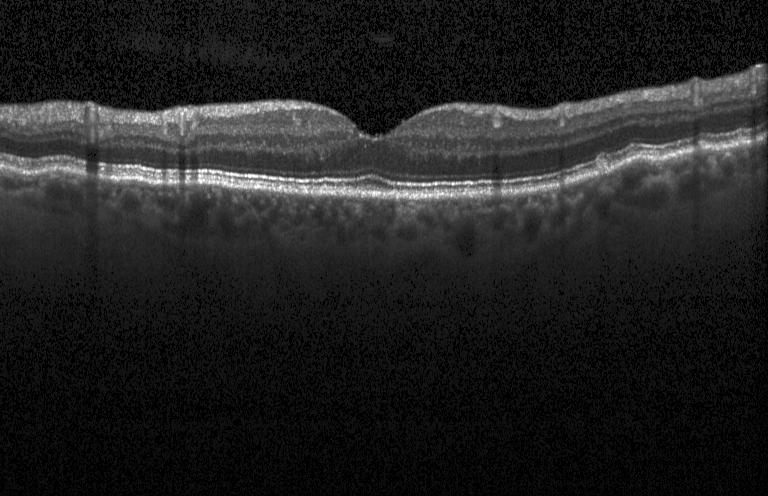

Diagnosis: drusen.